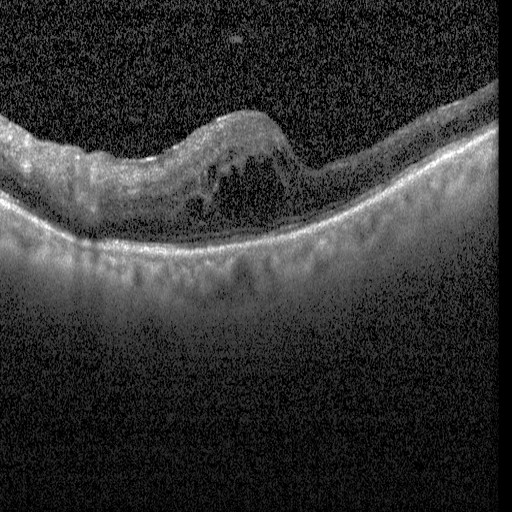
Retinal OCT cross-section showing DME.